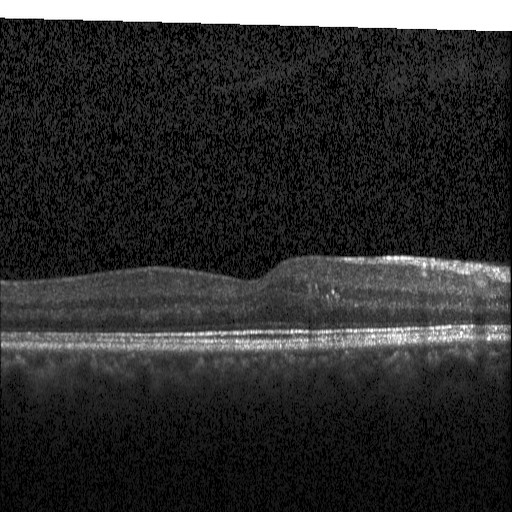
OCT line scan · macular scan · acquired on a Heidelberg Spectralis · SD-OCT — The scan shows DME.